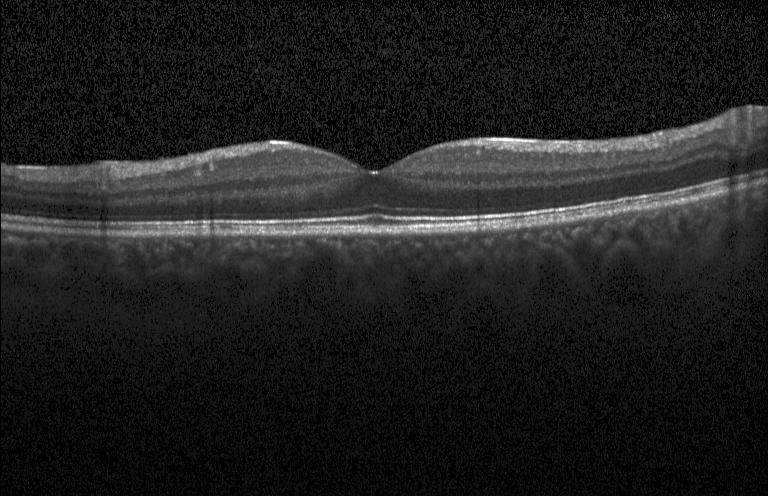
Retinal OCT cross-section. Diagnosis: no evidence of choroidal neovascularization, diabetic macular edema, or drusen.